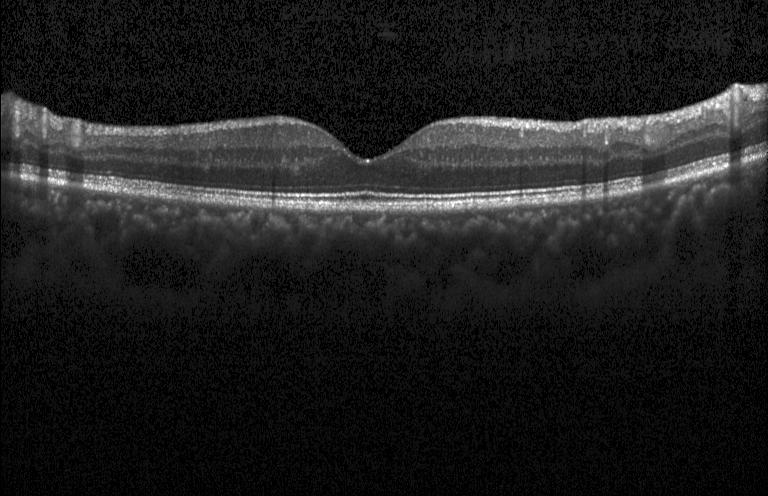

Heidelberg Spectralis OCT system; through the macula; SD-OCT; OCT line scan.
Macular OCT: no choroidal neovascularization, diabetic macular edema, or drusen.